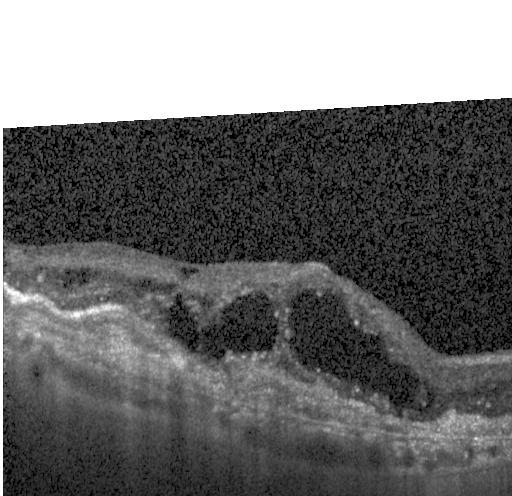 Diagnosis: a choroidal neovascular membrane.